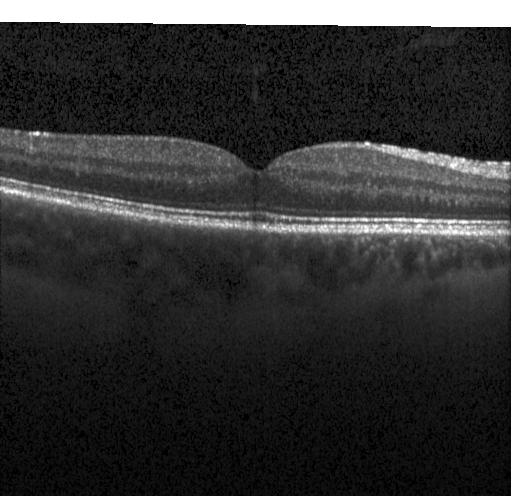 OCT B-scan · through the macula · spectral-domain optical coherence tomography · acquired on a Heidelberg Spectralis — Diagnosis: no evidence of choroidal neovascularization, diabetic macular edema, or drusen.